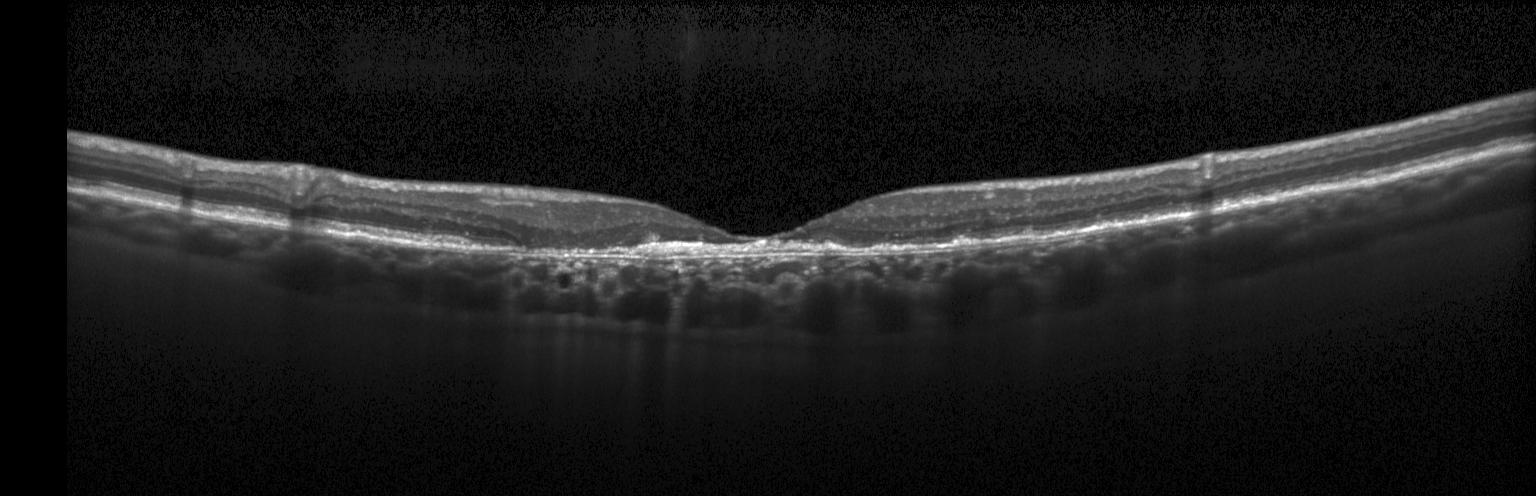
Spectral-domain optical coherence tomography · OCT line scan — Assessment: CNV.